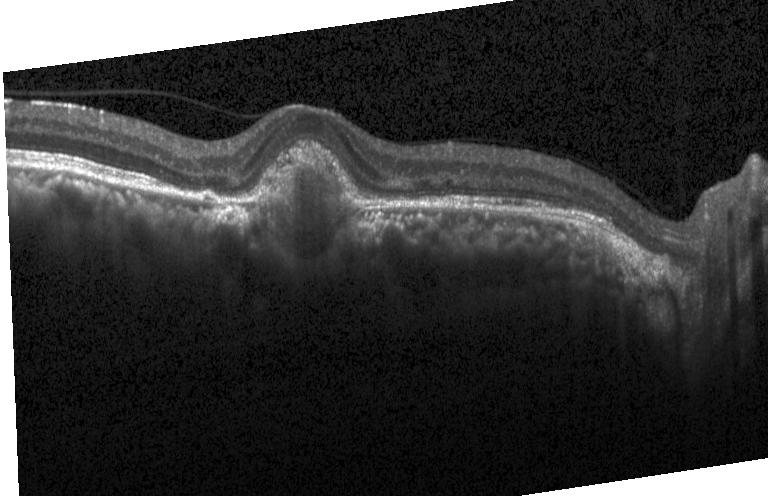

Optical coherence tomography B-scan; Heidelberg Spectralis OCT system — This B-scan demonstrates CNV.